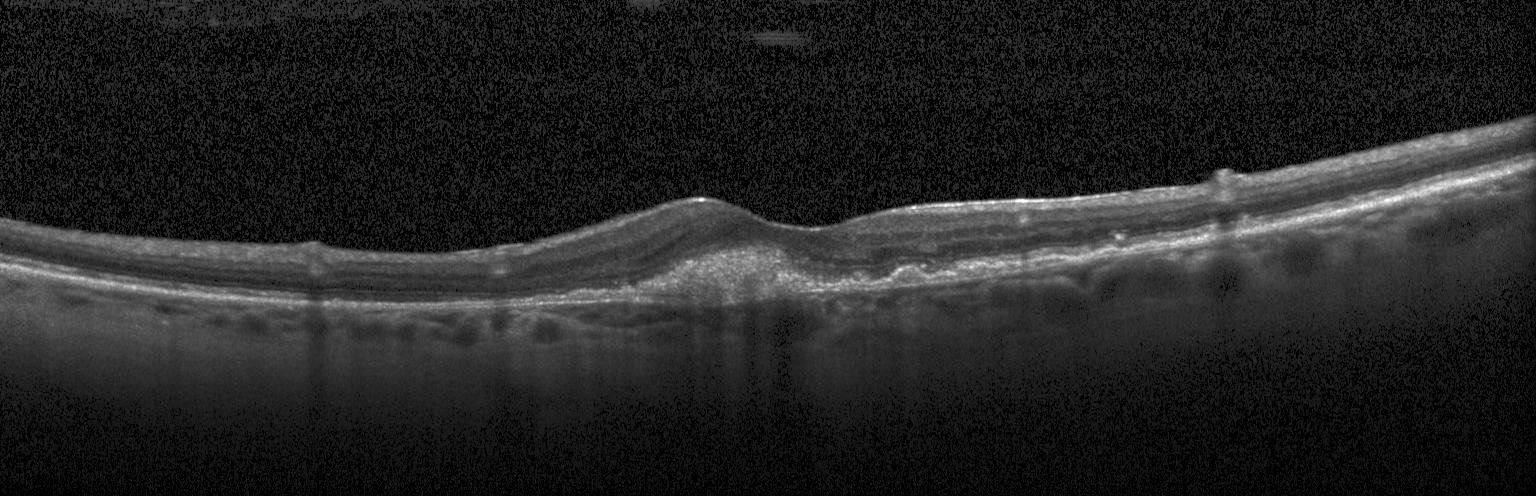 Impression: choroidal neovascularization.